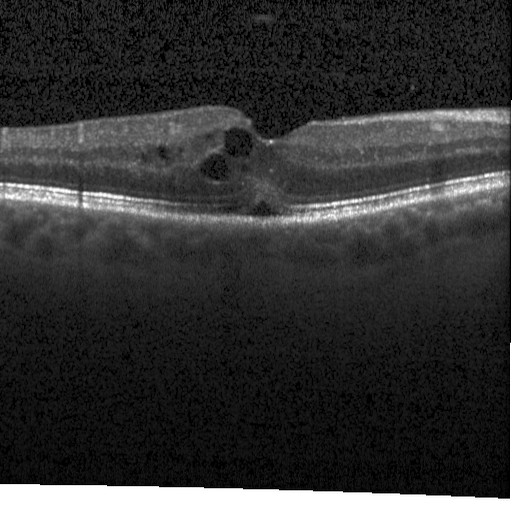
Spectral-domain OCT; optical coherence tomography scan; acquired on a Heidelberg Spectralis; centered on the fovea — Dx: diabetic macular edema (DME).